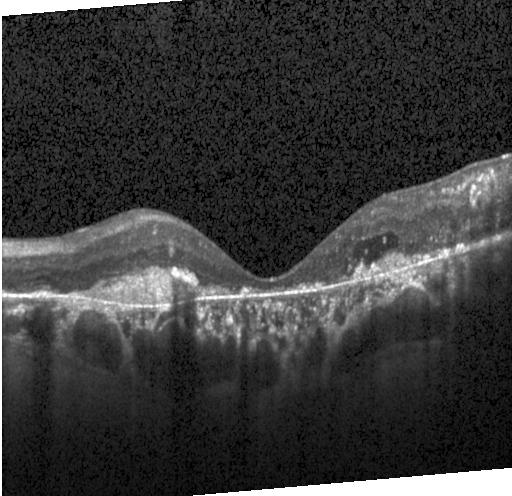 Heidelberg Spectralis OCT system · spectral-domain OCT · macular scan · OCT line scan
Impression: a choroidal neovascular membrane.